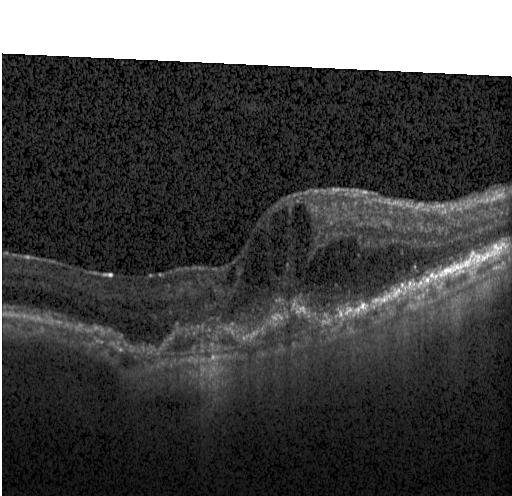 A choroidal neovascular membrane.